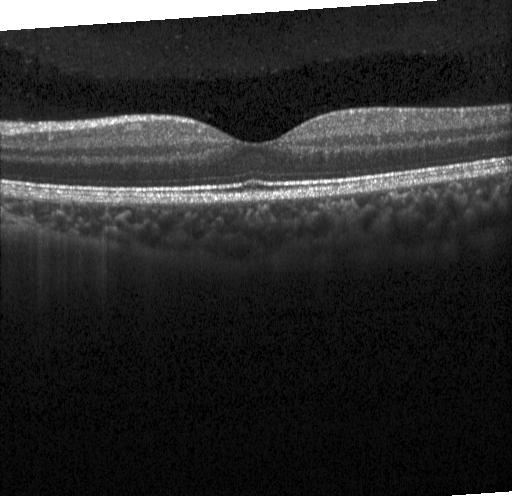
Through the macula, optical coherence tomography B-scan, Heidelberg Spectralis OCT system, spectral-domain OCT.
Impression: neither choroidal neovascularization, diabetic macular edema, nor drusen.